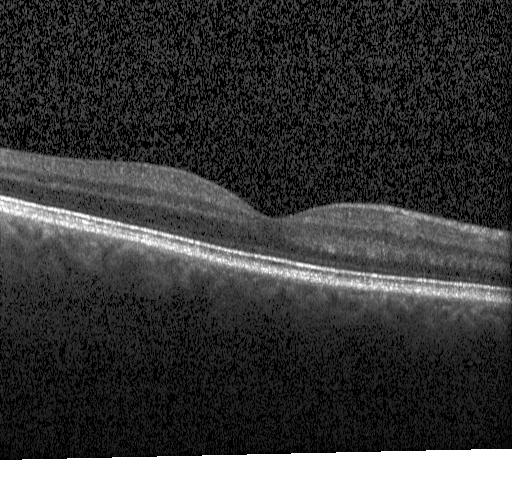

Retinal OCT B-scan; fovea-centered; acquired on a Heidelberg Spectralis.
Diagnosis: no evidence of choroidal neovascularization, diabetic macular edema, or drusen.